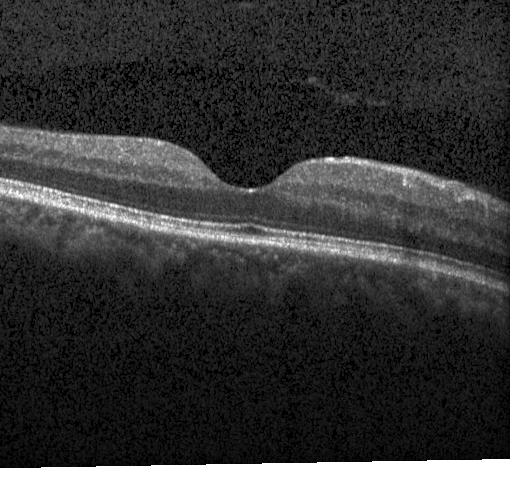
OCT scan showing no choroidal neovascularization, diabetic macular edema, or drusen.